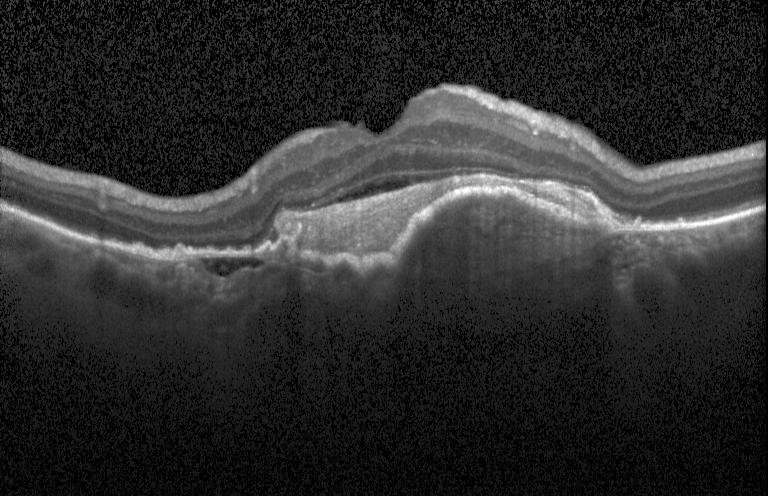 Retinal OCT cross-section, spectral-domain OCT — Macular OCT: a choroidal neovascular membrane.